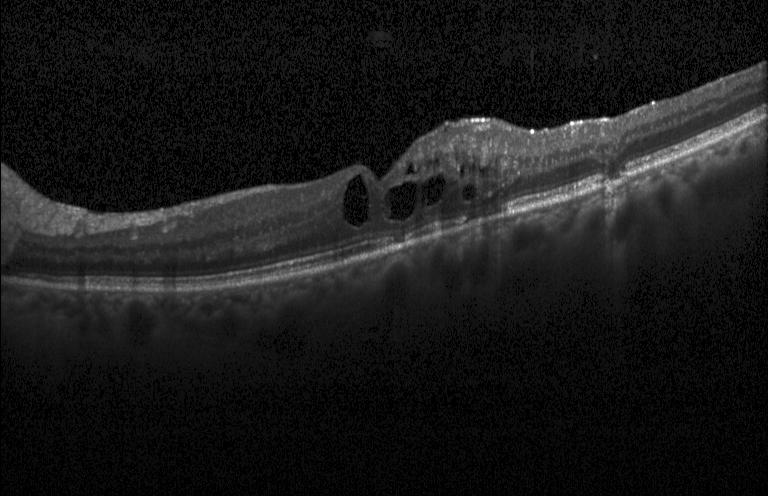
Centered on the fovea · SD-OCT · OCT line scan
Assessment: DME.